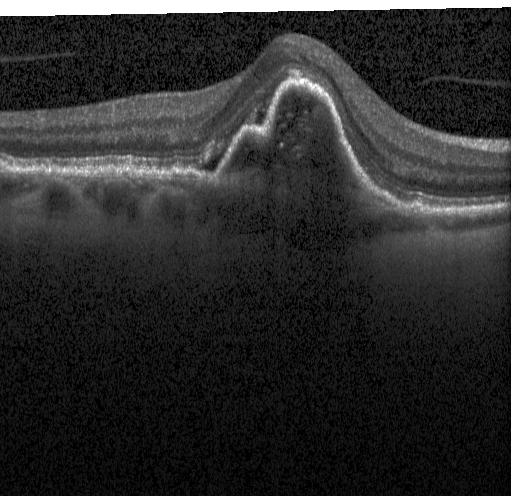
Retinal OCT cross-section showing CNV.